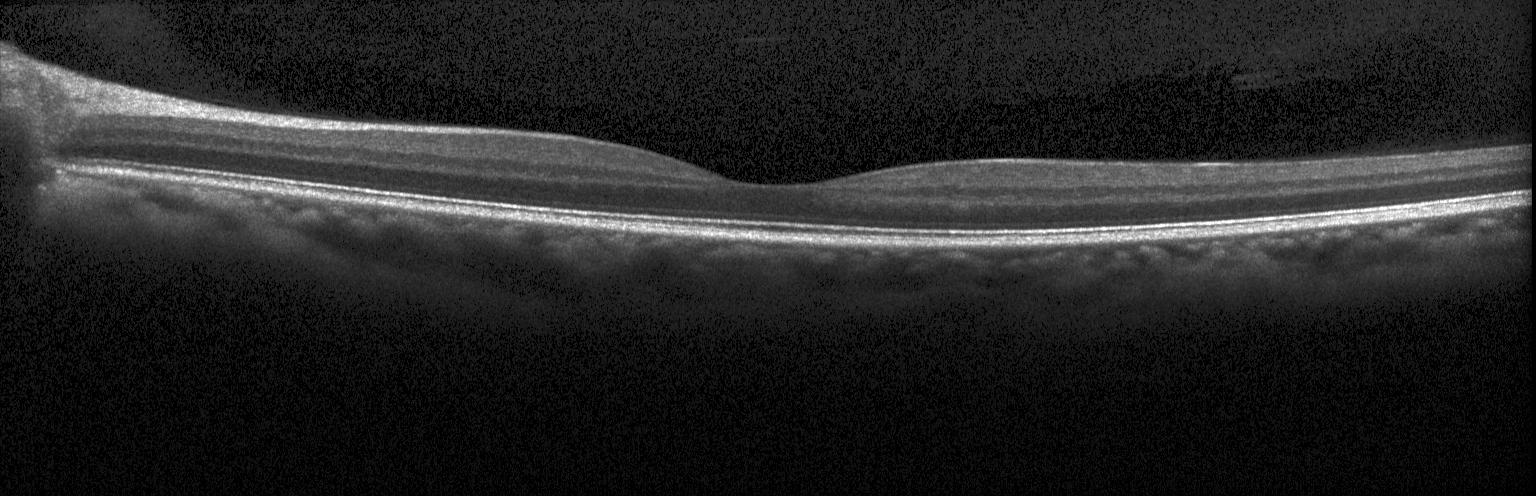
Impression: neither choroidal neovascularization, diabetic macular edema, nor drusen.